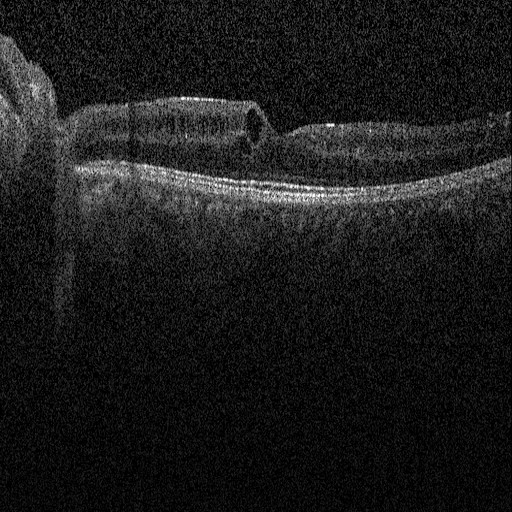
Through the macula, retinal OCT cross-section, spectral-domain optical coherence tomography.
Impression: diabetic macular edema (DME).